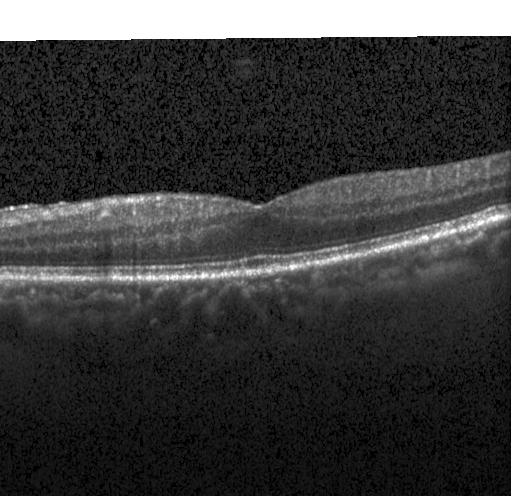
OCT B-scan.
Dx: neither choroidal neovascularization, diabetic macular edema, nor drusen.